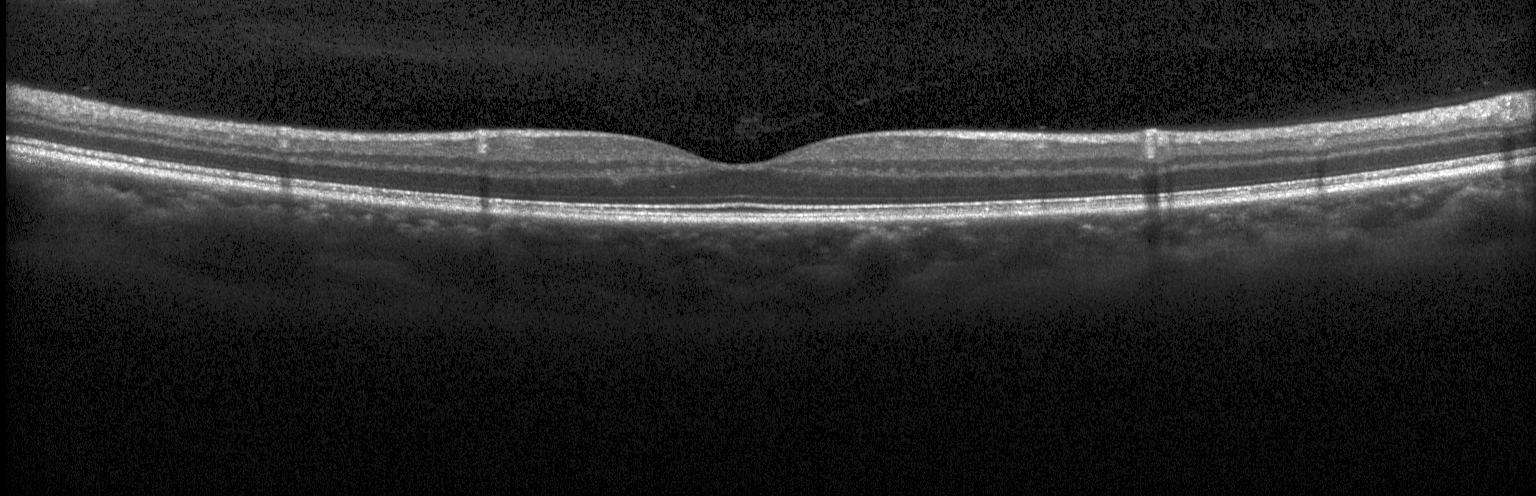
Optical coherence tomography B-scan. OCT finding: no choroidal neovascularization, diabetic macular edema, or drusen.